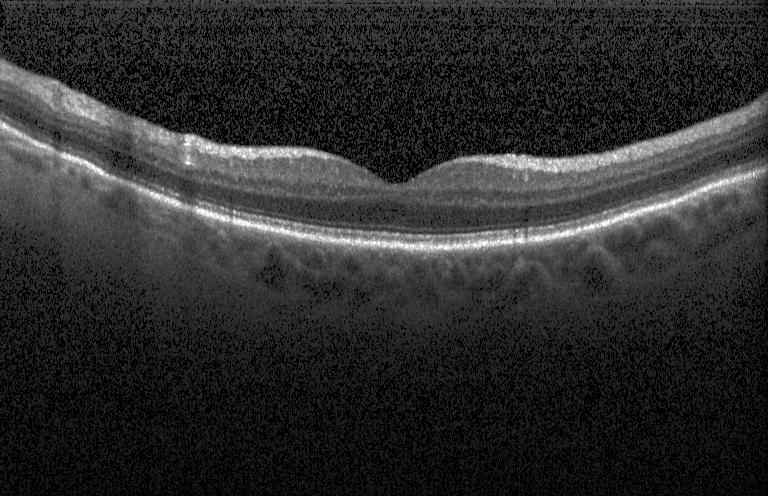
Optical coherence tomography B-scan. Diagnosis: neither CNV, DME, nor drusen.